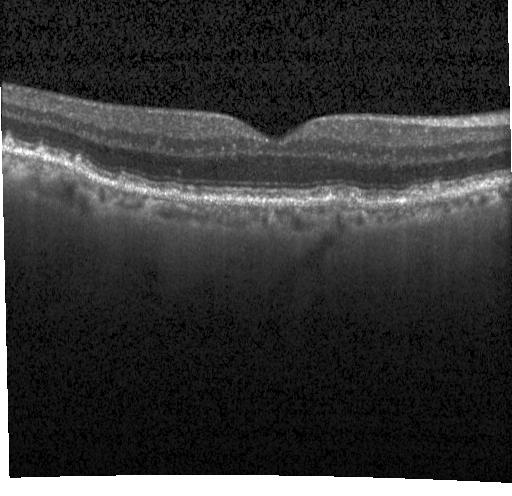

Optical coherence tomography scan. Through the macula. Spectral-domain optical coherence tomography
The scan shows drusen.